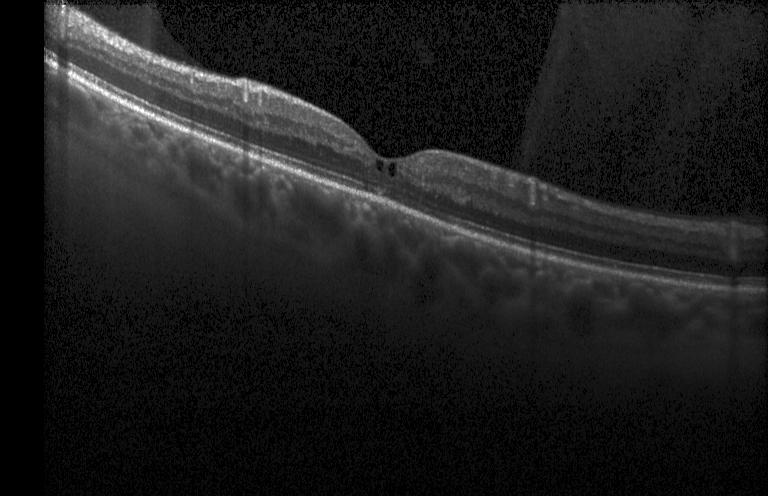
The scan shows diabetic macular edema (DME).